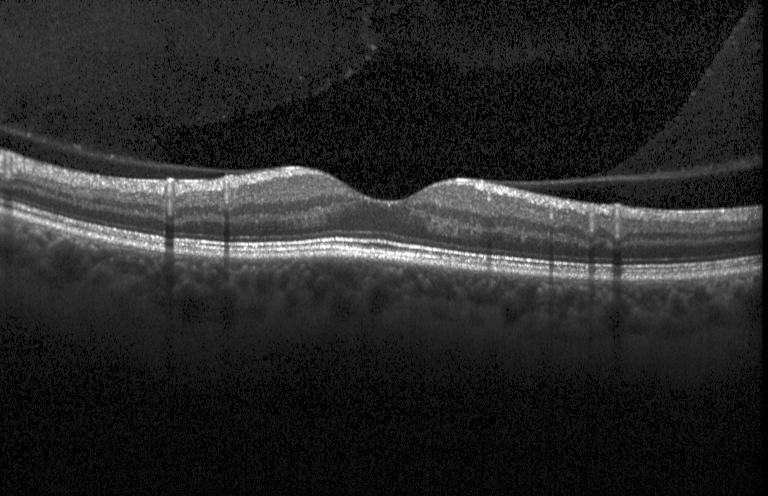 Diagnosis: neither choroidal neovascularization, diabetic macular edema, nor drusen.